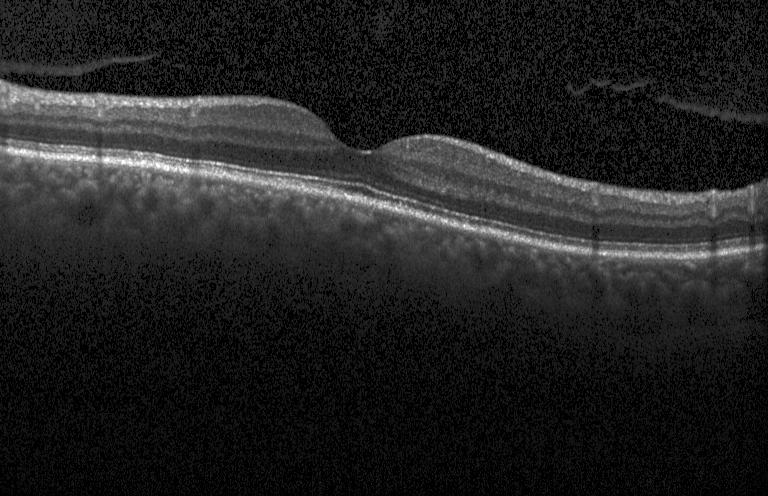
Optical coherence tomography scan
This B-scan demonstrates no choroidal neovascularization, no diabetic macular edema, and no drusen.